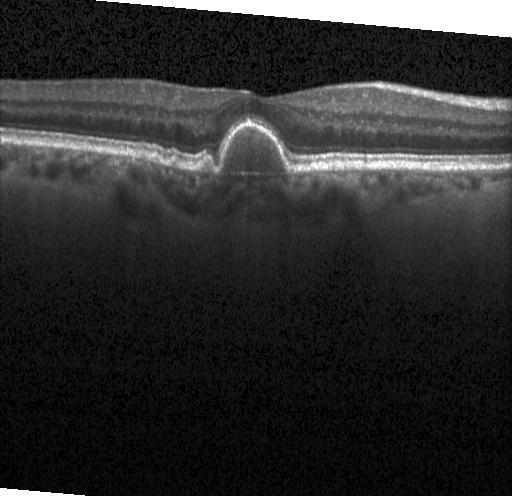

Diagnosis: CNV.